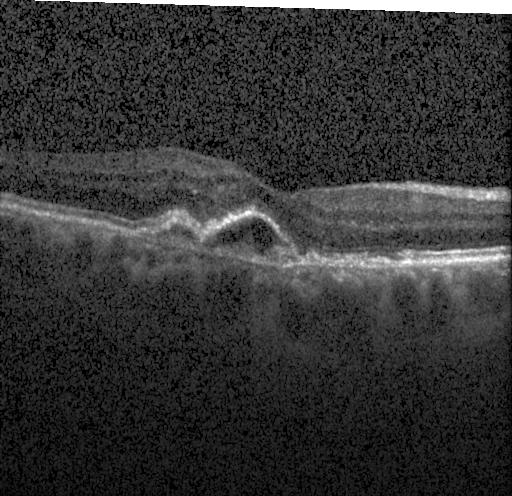

Optical coherence tomography scan · horizontal scan through the fovea · Heidelberg Spectralis OCT system · spectral-domain OCT — A choroidal neovascular membrane.